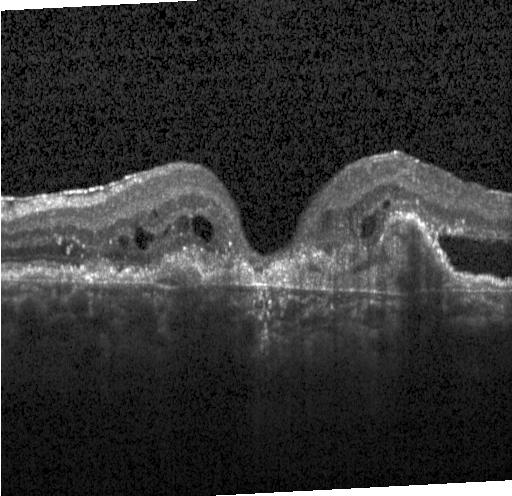 Impression: a choroidal neovascular membrane.